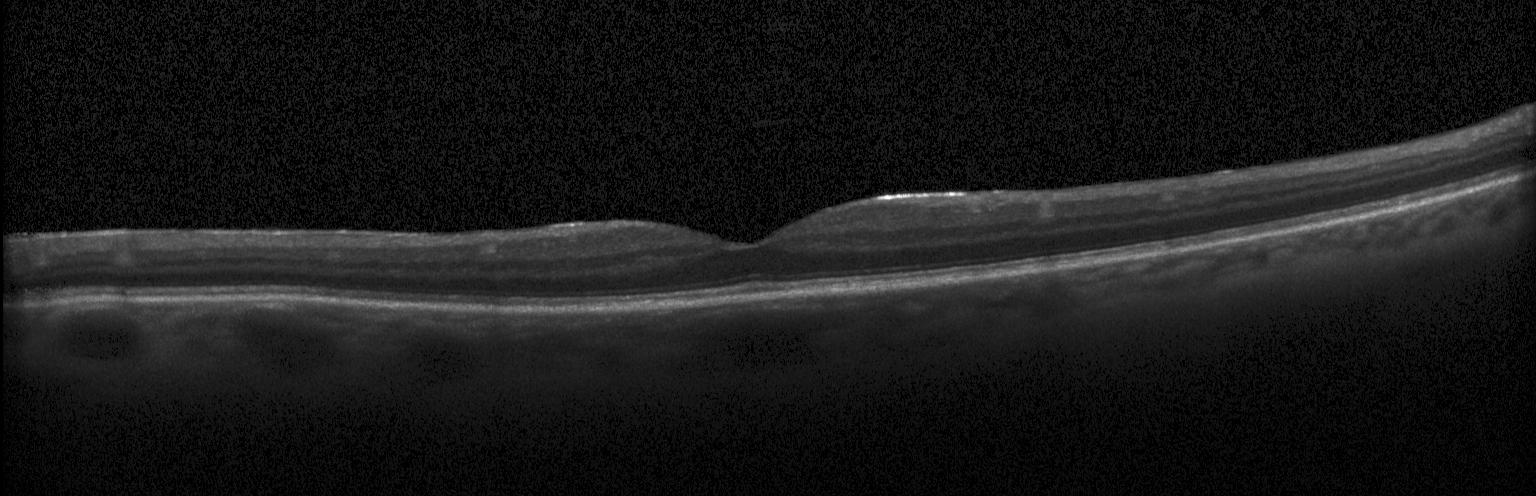 Macular OCT demonstrating no choroidal neovascularization, diabetic macular edema, or drusen.